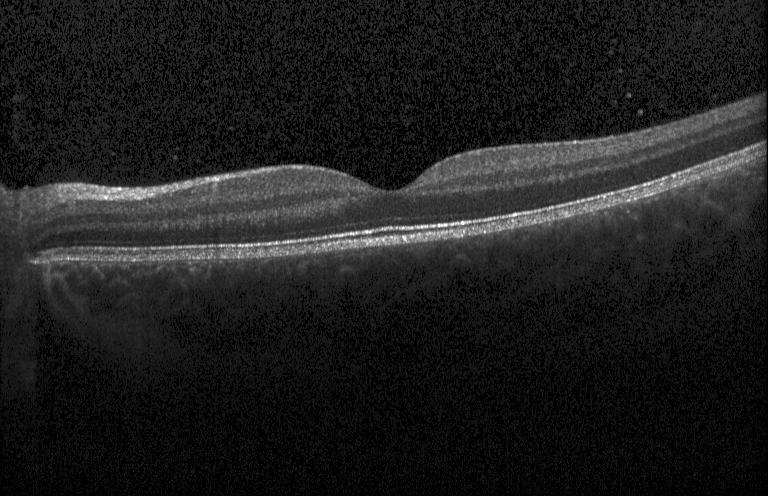 OCT scan showing no evidence of choroidal neovascularization, diabetic macular edema, or drusen.